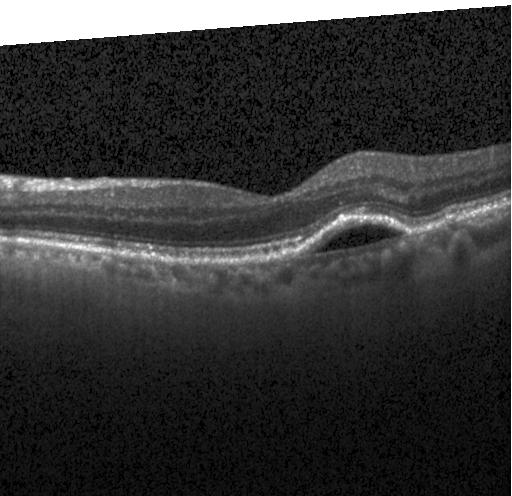 Optical coherence tomography B-scan; Heidelberg Spectralis; macular scan
Diagnosis: choroidal neovascularization.